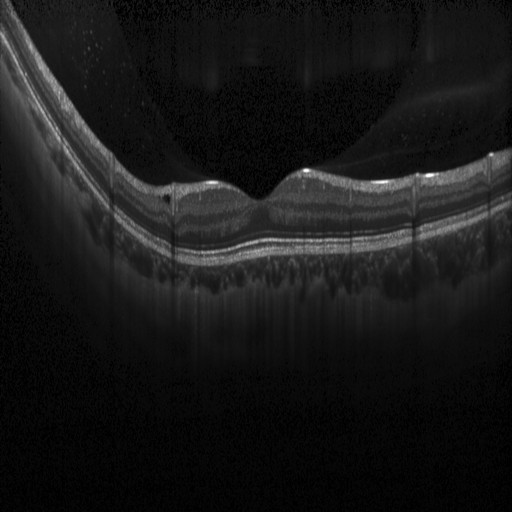 Macular OCT: diabetic macular edema.